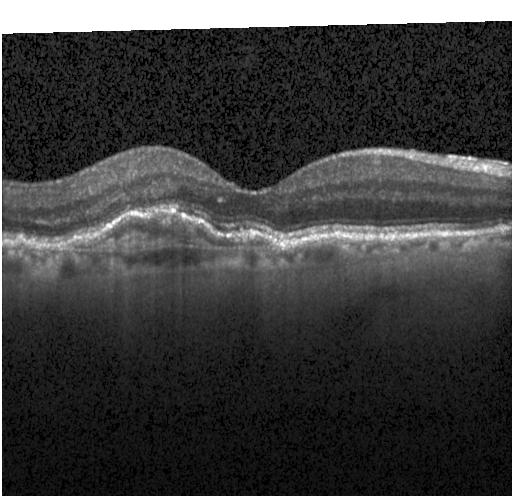 OCT line scan. Fovea-centered. SD-OCT. Diagnosis: a choroidal neovascular membrane.